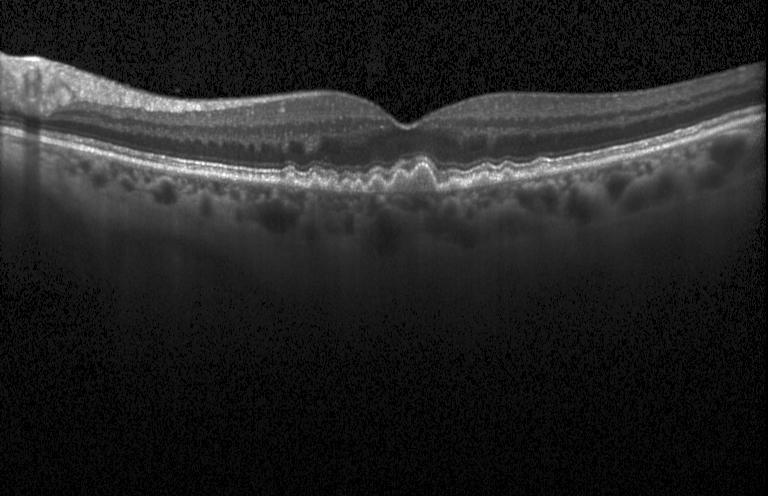
Heidelberg Spectralis OCT system, OCT B-scan, macular scan
Macular OCT: drusen.